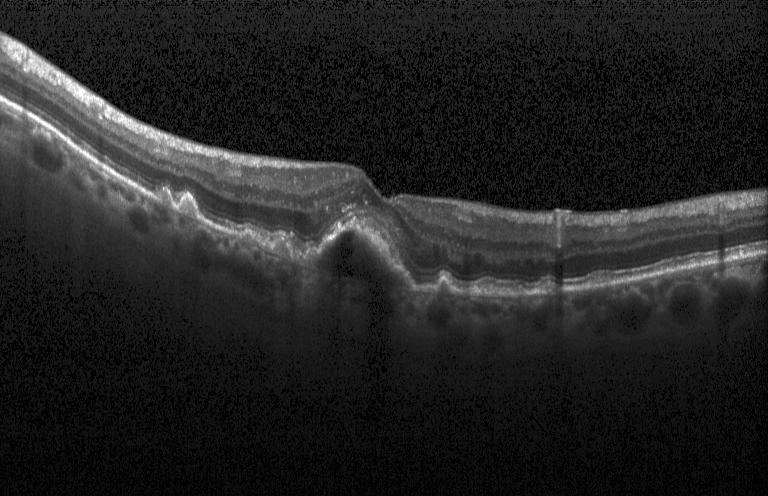 SD-OCT · OCT line scan · Heidelberg Spectralis.
CNV.